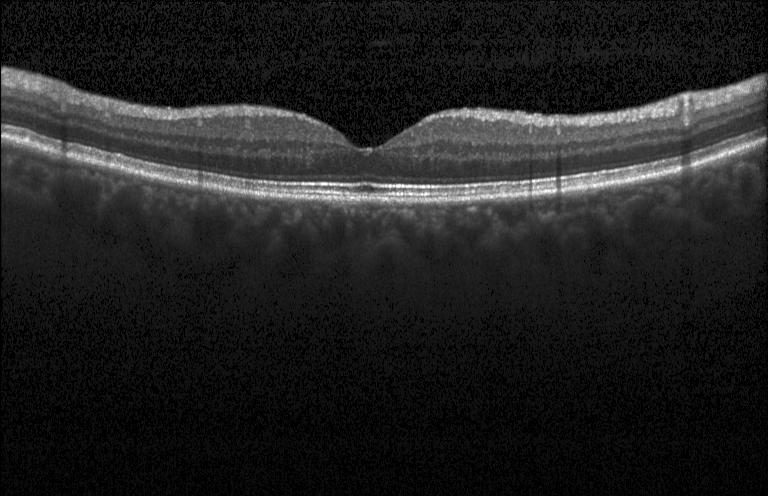 OCT B-scan; through the macula
Dx: no choroidal neovascularization, no diabetic macular edema, and no drusen.